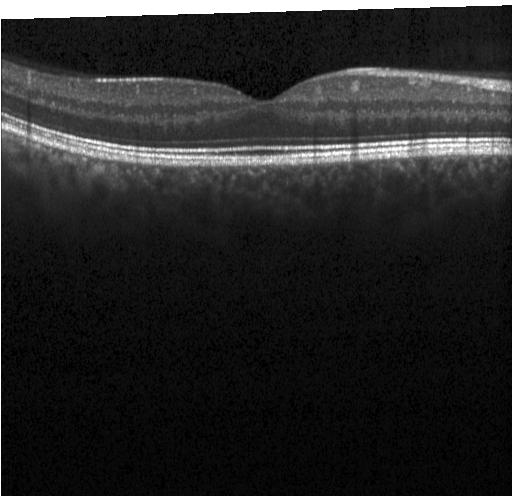
Centered on the fovea; acquired on a Heidelberg Spectralis; OCT line scan. Impression: no choroidal neovascularization, no diabetic macular edema, and no drusen.